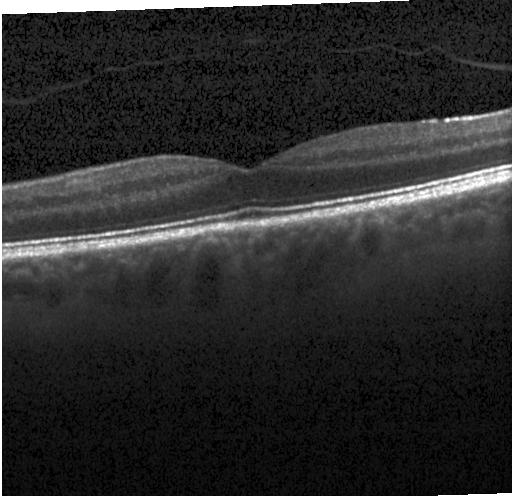 Macular OCT demonstrating no evidence of choroidal neovascularization, diabetic macular edema, or drusen.